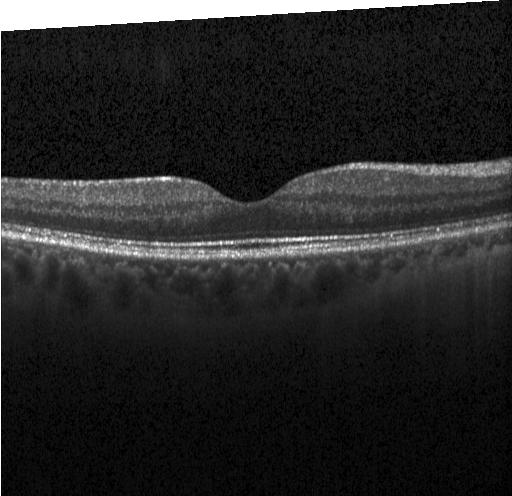
Instrument: Heidelberg Spectralis · spectral-domain OCT · retinal OCT B-scan. This B-scan demonstrates neither choroidal neovascularization, diabetic macular edema, nor drusen.